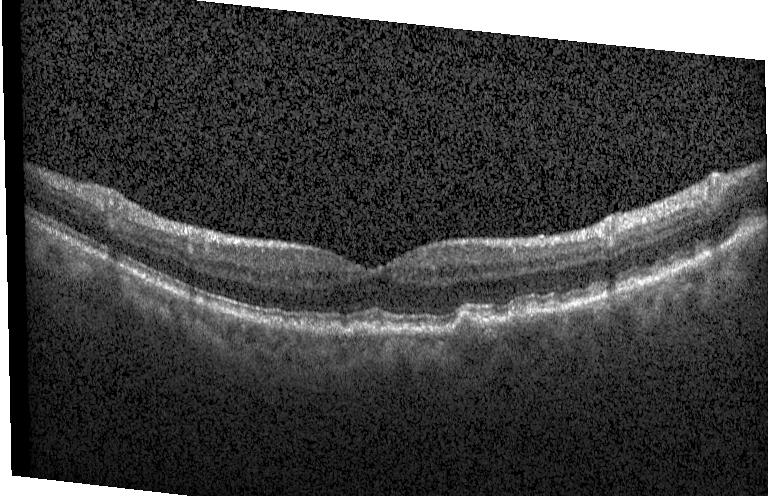
OCT line scan. Heidelberg Spectralis. Spectral-domain optical coherence tomography
Macular OCT: multiple drusen.